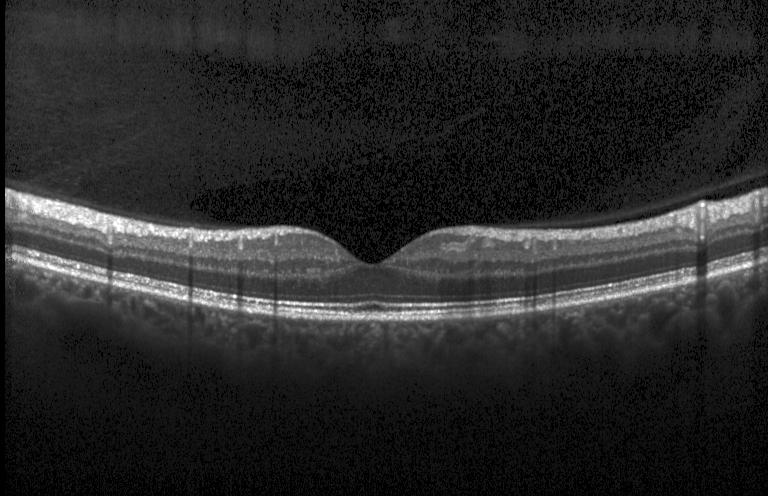

OCT finding: no choroidal neovascularization, diabetic macular edema, or drusen.